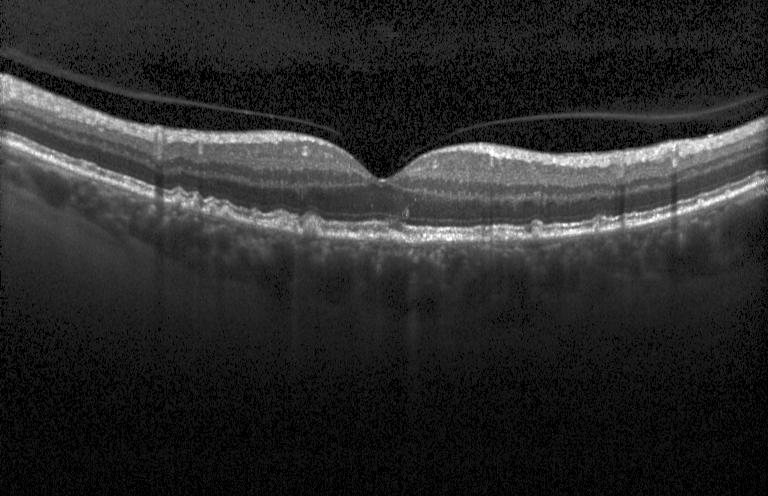

Retinal OCT B-scan.
Macular OCT: sub-RPE drusenoid deposits.